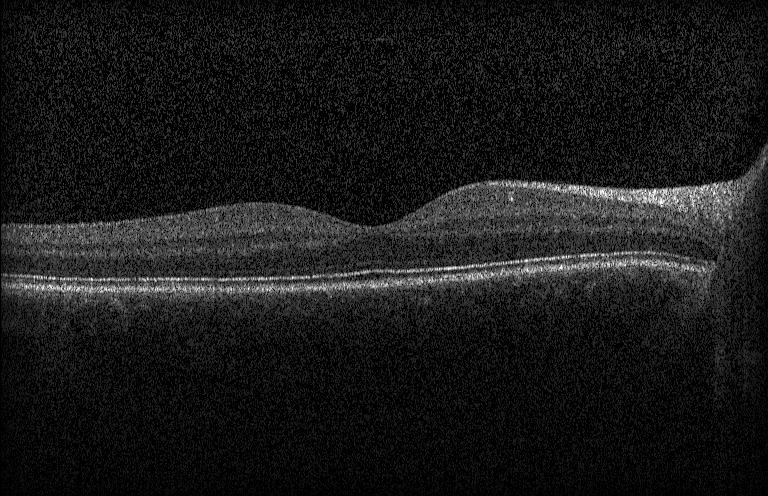

Acquired on a Heidelberg Spectralis · optical coherence tomography scan — No choroidal neovascularization, diabetic macular edema, or drusen.